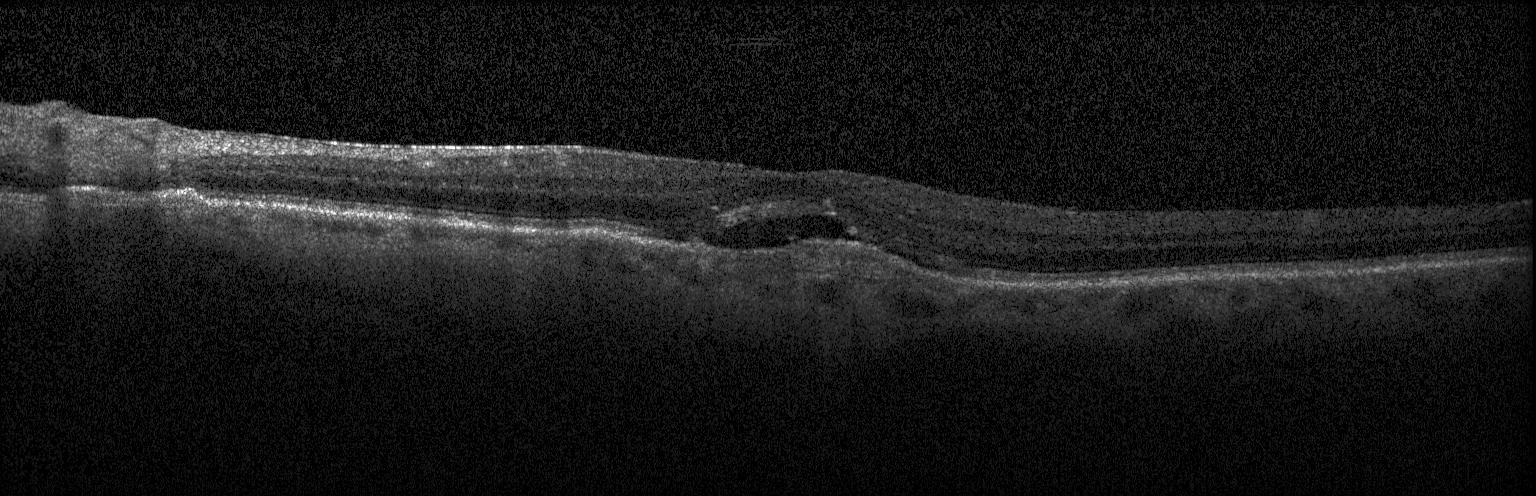

OCT B-scan showing a choroidal neovascular membrane.